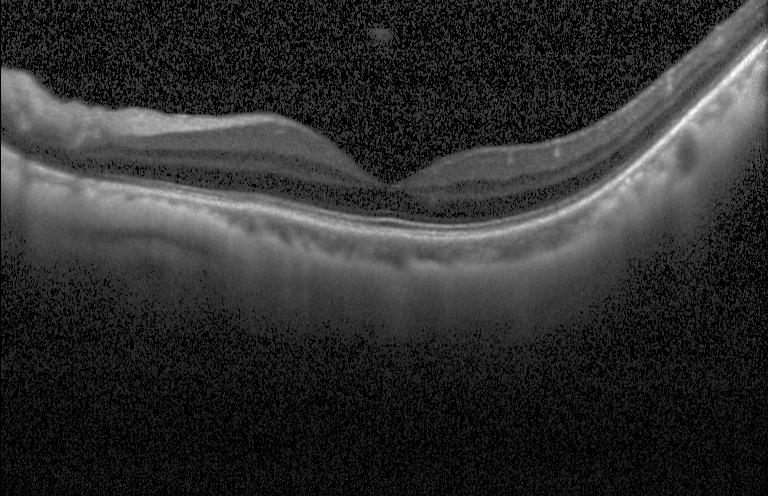 Spectral-domain OCT; macular scan; OCT line scan; acquired on a Heidelberg Spectralis — OCT finding: no evidence of choroidal neovascularization, diabetic macular edema, or drusen.